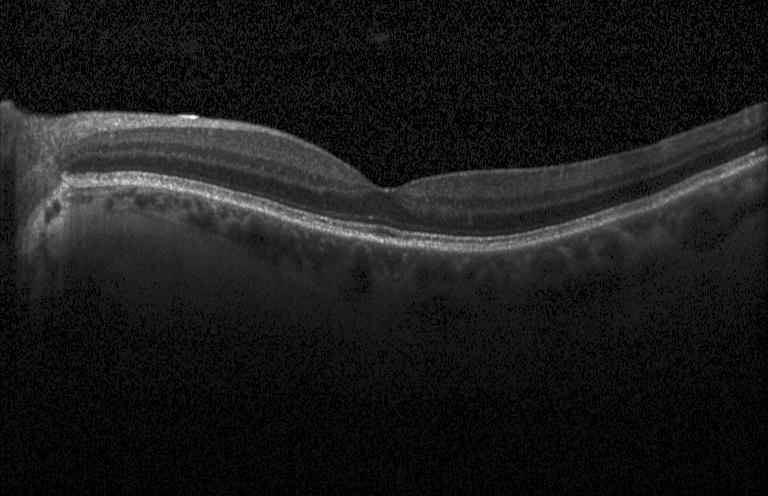
OCT line scan. Macular OCT: no choroidal neovascularization, no diabetic macular edema, and no drusen.